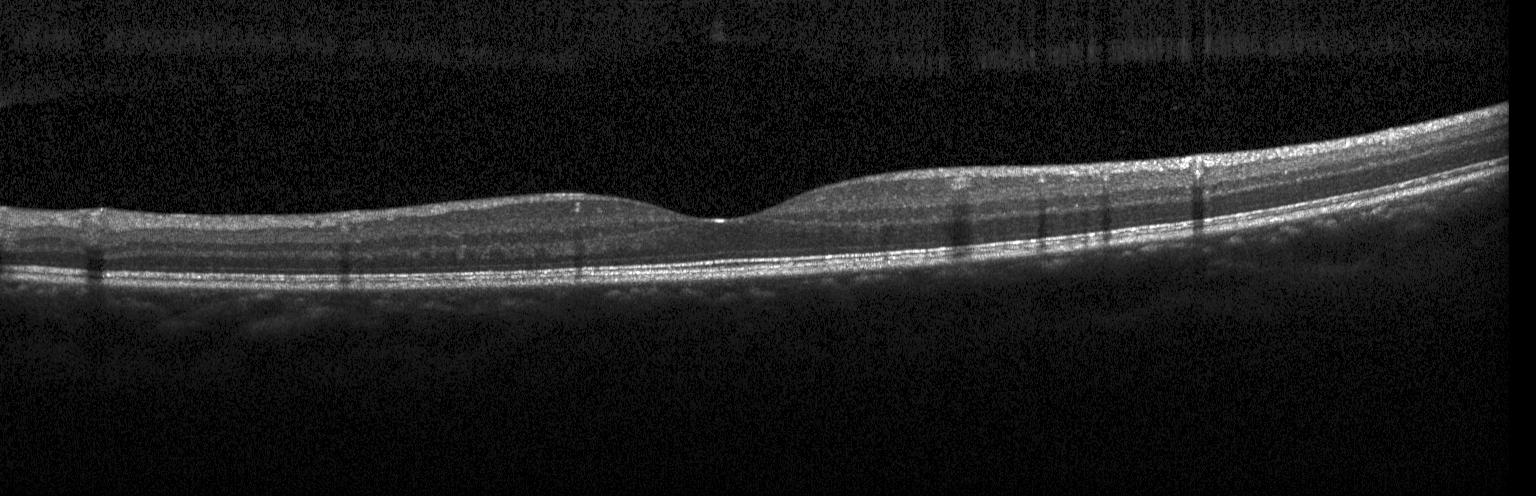

Retinal OCT B-scan.
Finding: no choroidal neovascularization, diabetic macular edema, or drusen.